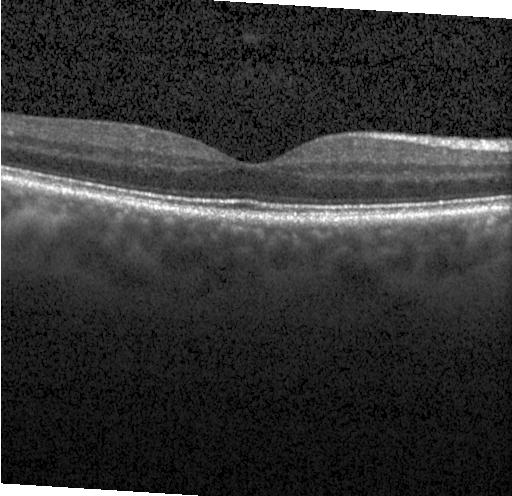
SD-OCT. Optical coherence tomography scan. No evidence of choroidal neovascularization, diabetic macular edema, or drusen.